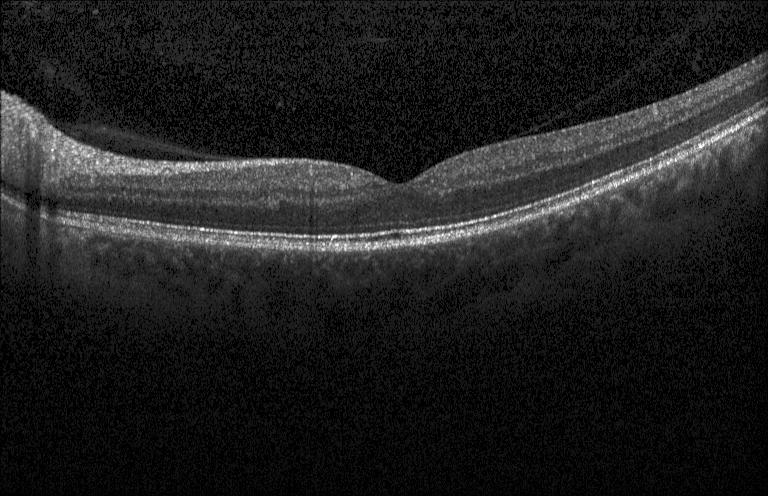

Acquired on a Heidelberg Spectralis, through the macula, SD-OCT, retinal OCT B-scan
Assessment: no CNV, no DME, and no drusen.